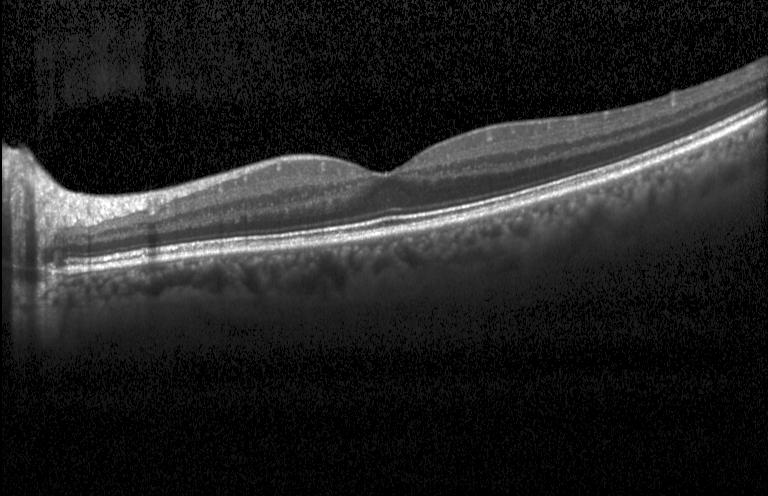

Impression: no evidence of choroidal neovascularization, diabetic macular edema, or drusen.